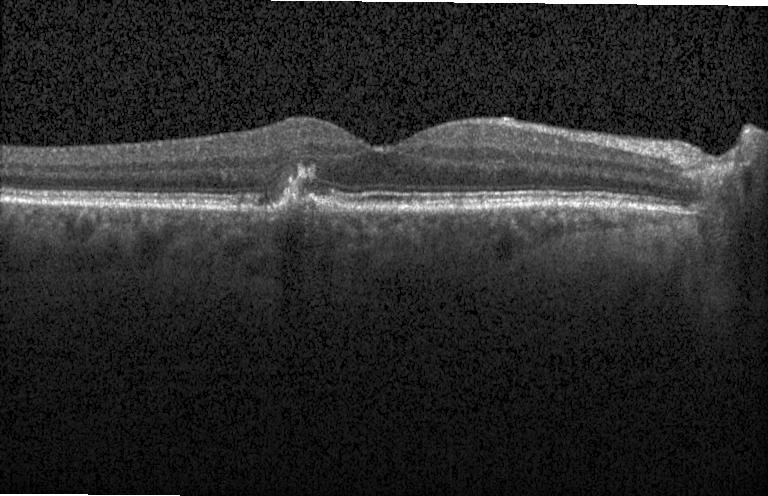

Finding: a choroidal neovascular membrane.